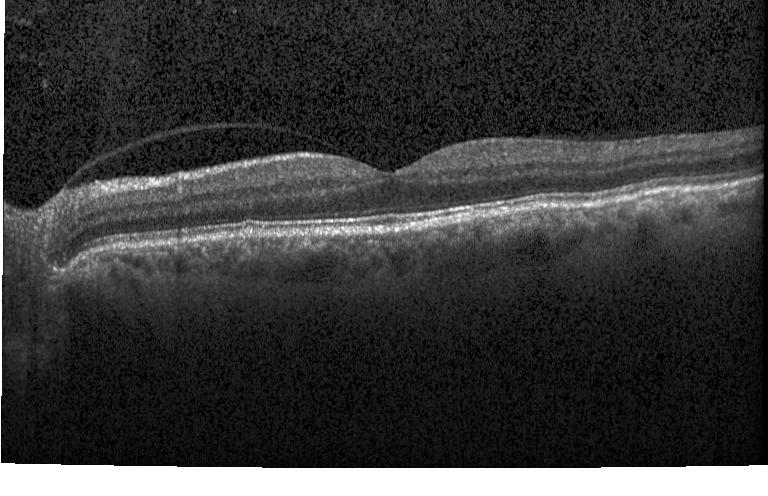 Impression: no evidence of CNV, DME, or drusen.